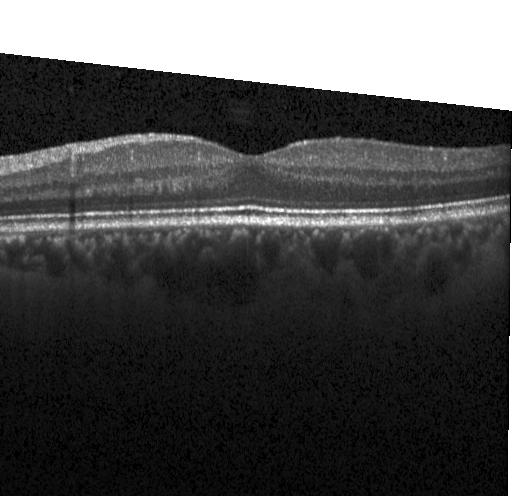
Spectral-domain optical coherence tomography, Heidelberg Spectralis OCT system, retinal OCT cross-section, centered on the fovea
Diagnosis: no evidence of choroidal neovascularization, diabetic macular edema, or drusen.